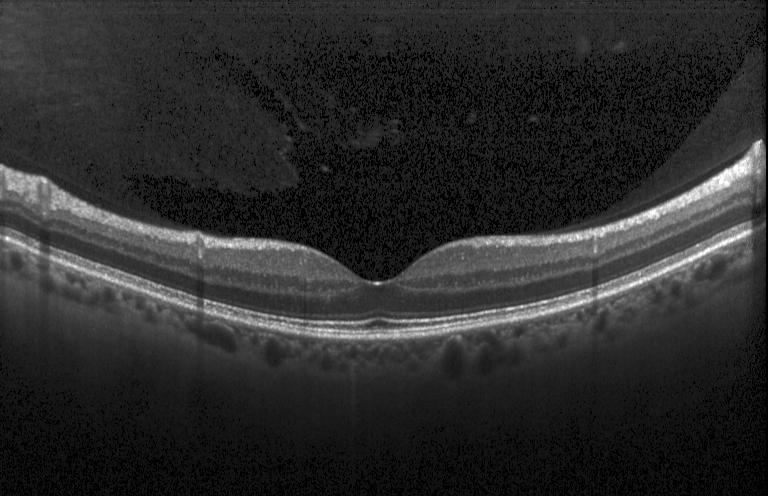
Diagnosis: no choroidal neovascularization, diabetic macular edema, or drusen.